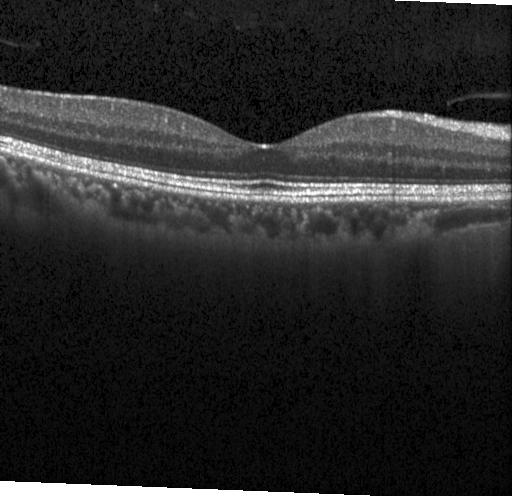

Optical coherence tomography B-scan, spectral-domain optical coherence tomography, centered on the fovea, Heidelberg Spectralis — Diagnosis: no choroidal neovascularization, no diabetic macular edema, and no drusen.